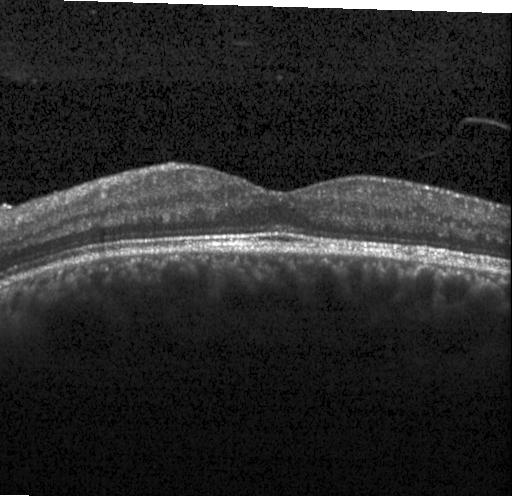

Optical coherence tomography scan; spectral-domain OCT; horizontal scan through the fovea.
OCT finding: neither choroidal neovascularization, diabetic macular edema, nor drusen.